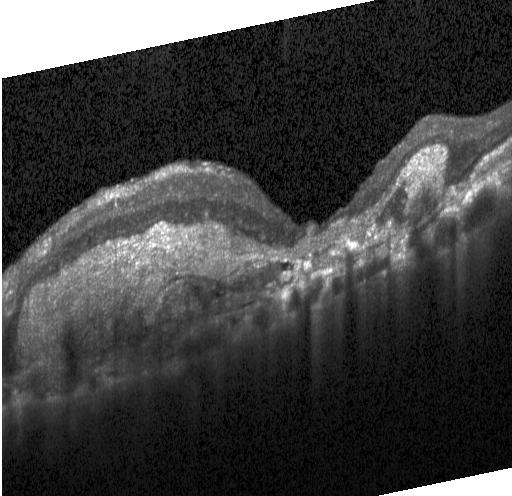

Macular OCT: a choroidal neovascular membrane.